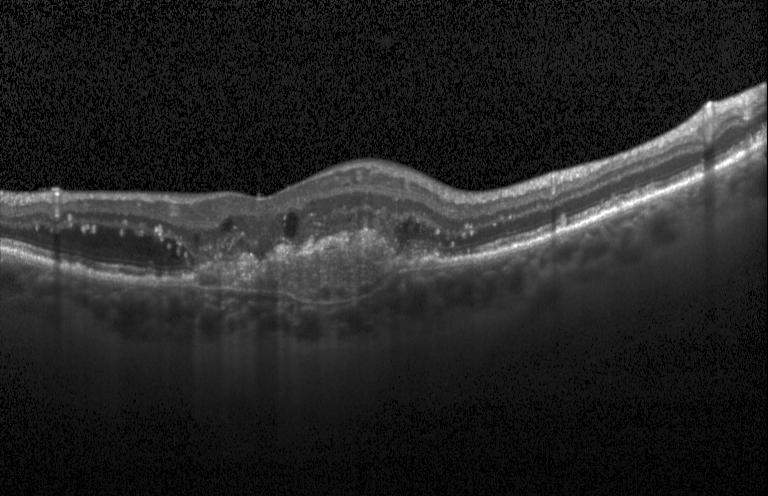
Dx: CNV.